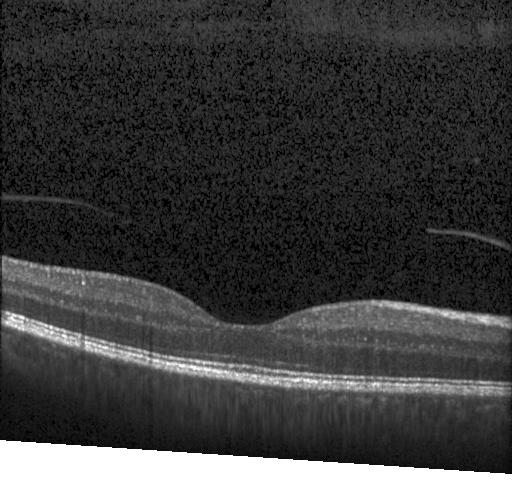

Retinal OCT B-scan, instrument: Heidelberg Spectralis, macular scan. OCT finding: no evidence of choroidal neovascularization, diabetic macular edema, or drusen.